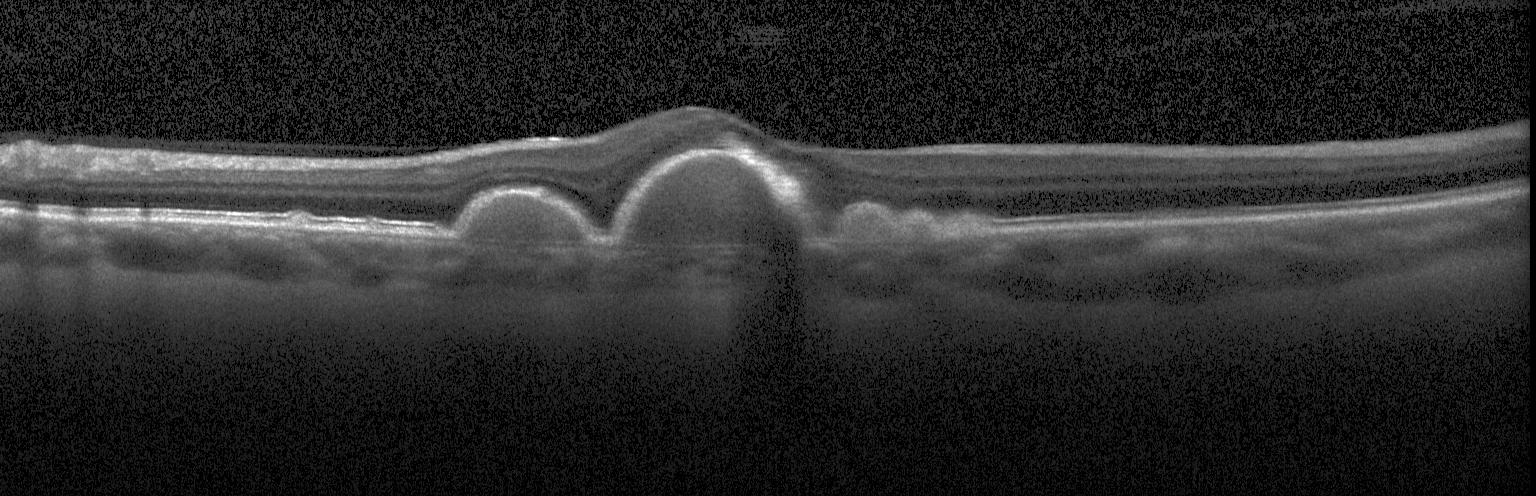 Impression: a choroidal neovascular membrane.